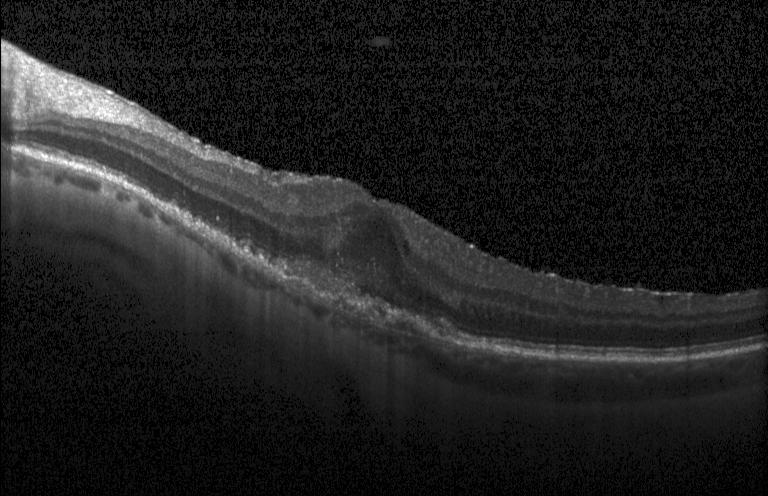

Impression: a choroidal neovascular membrane.